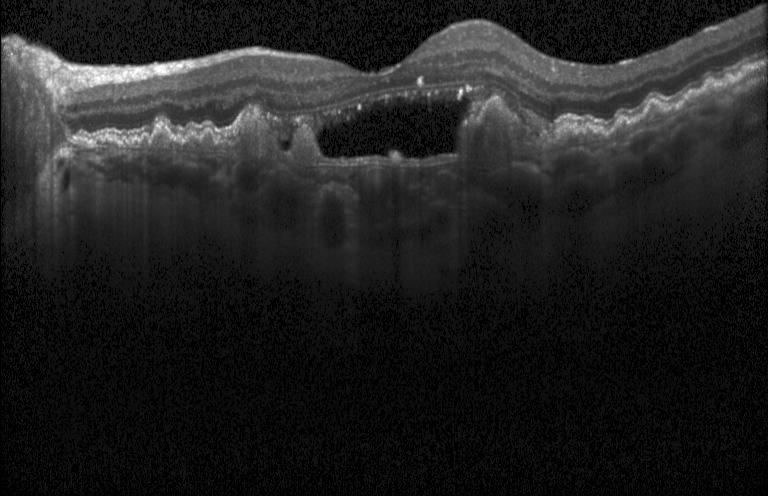

Spectral-domain OCT B-scan: choroidal neovascularization.